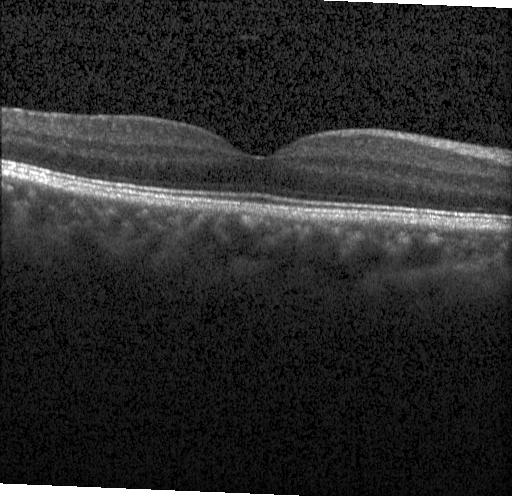 Retinal OCT B-scan
Assessment: no choroidal neovascularization, no diabetic macular edema, and no drusen.